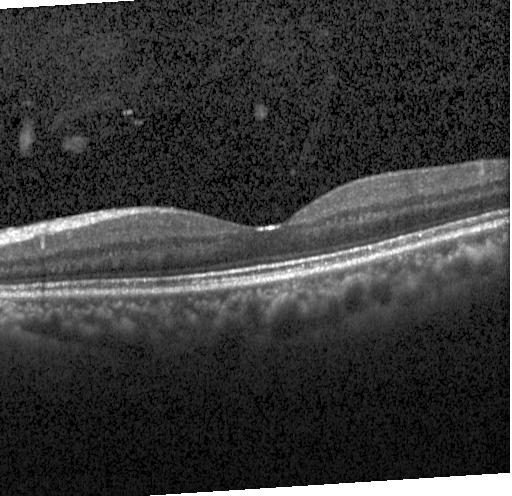
Retinal OCT B-scan; macular scan.
The scan shows neither CNV, DME, nor drusen.